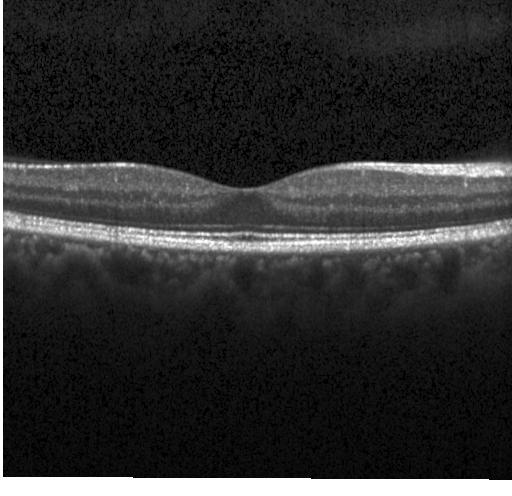 Optical coherence tomography B-scan — Diagnosis: neither choroidal neovascularization, diabetic macular edema, nor drusen.